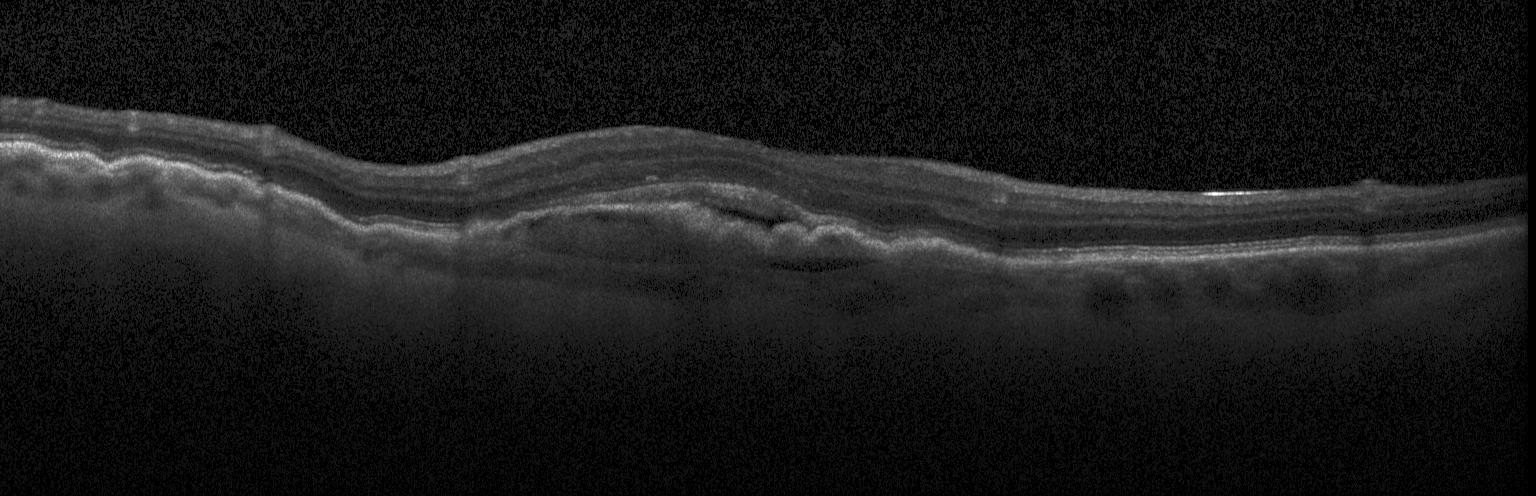

Heidelberg Spectralis · macular scan · OCT B-scan · SD-OCT — The scan shows choroidal neovascularization.